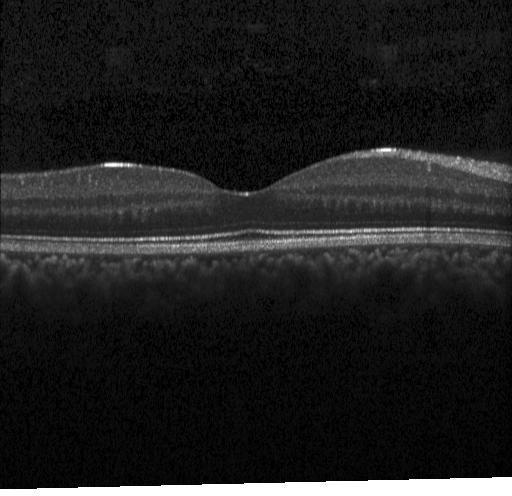
OCT B-scan, SD-OCT
This B-scan demonstrates no CNV, DME, or drusen.